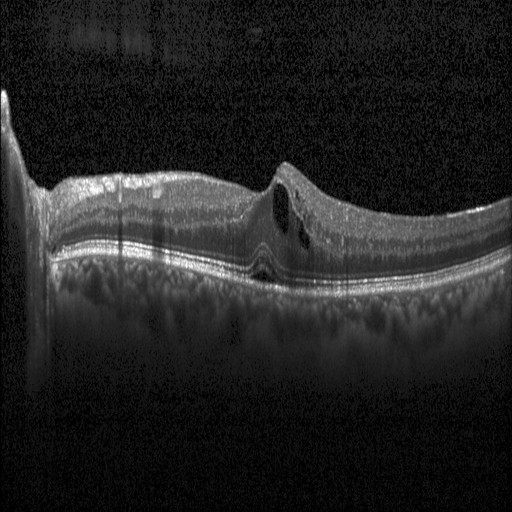
Retinal OCT cross-section
Finding: diabetic macular edema.